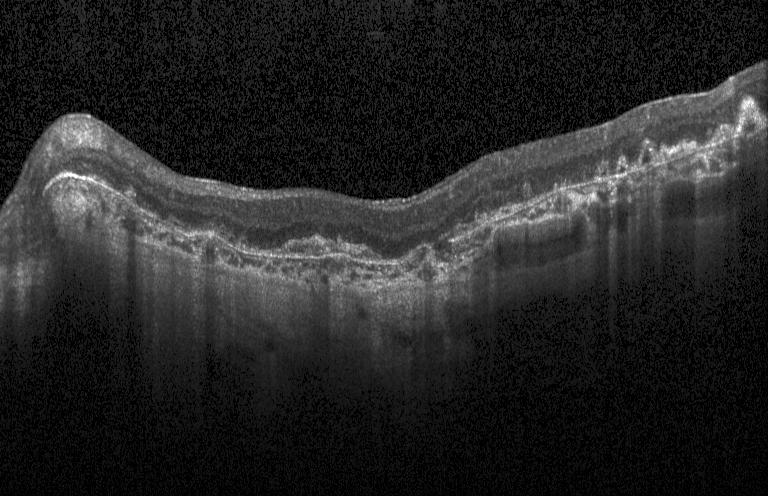

Retinal OCT B-scan. Acquired on a Heidelberg Spectralis. Centered on the fovea
Finding: choroidal neovascularization.